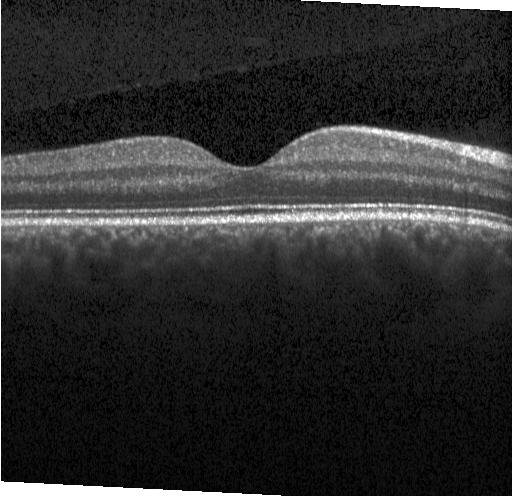
Impression: neither CNV, DME, nor drusen.